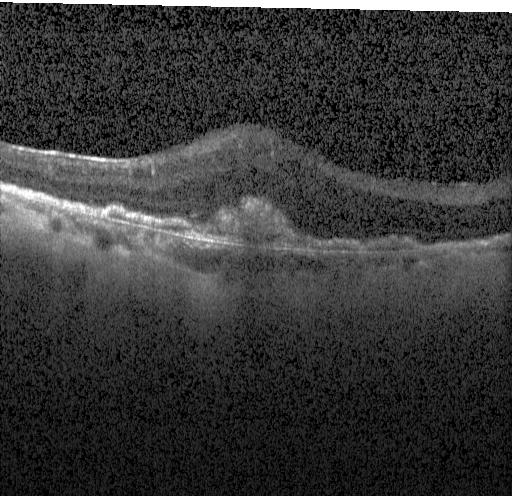 Optical coherence tomography B-scan — A choroidal neovascular membrane.